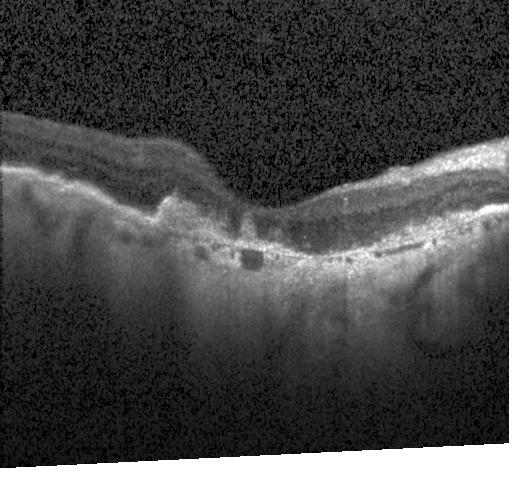
Macular OCT demonstrating a choroidal neovascular membrane.